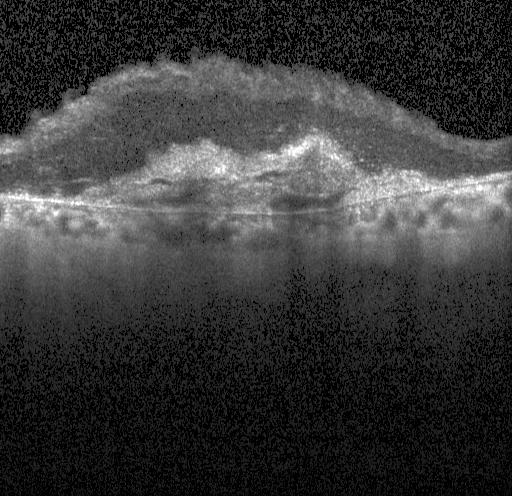 Fovea-centered; Heidelberg Spectralis; spectral-domain OCT; retinal OCT cross-section
Assessment: a choroidal neovascular membrane.